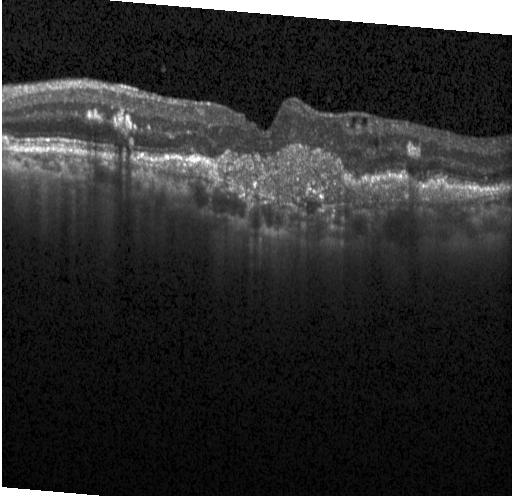
Diagnosis: a choroidal neovascular membrane.